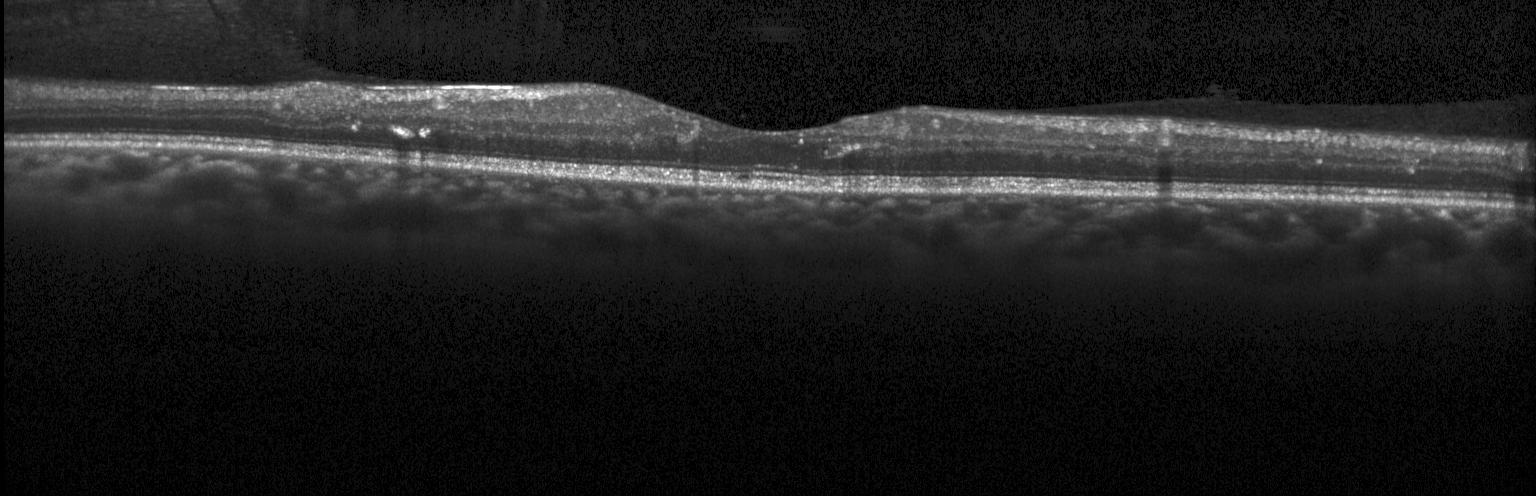

Finding: DME.